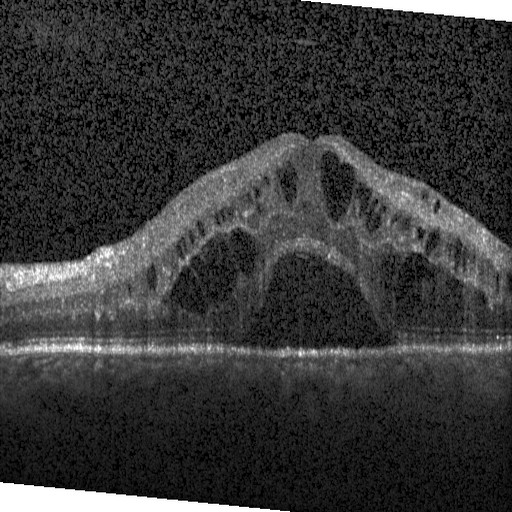
Retinal OCT cross-section. Spectral-domain OCT — Finding: diabetic macular edema (DME).